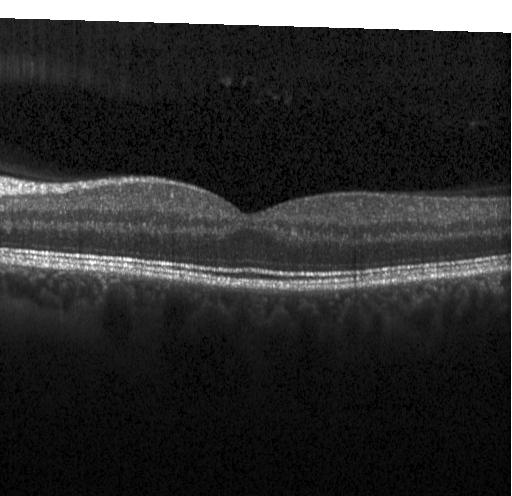
Through the macula. Spectral-domain OCT. Heidelberg Spectralis. Optical coherence tomography B-scan
Diagnosis: no choroidal neovascularization, diabetic macular edema, or drusen.